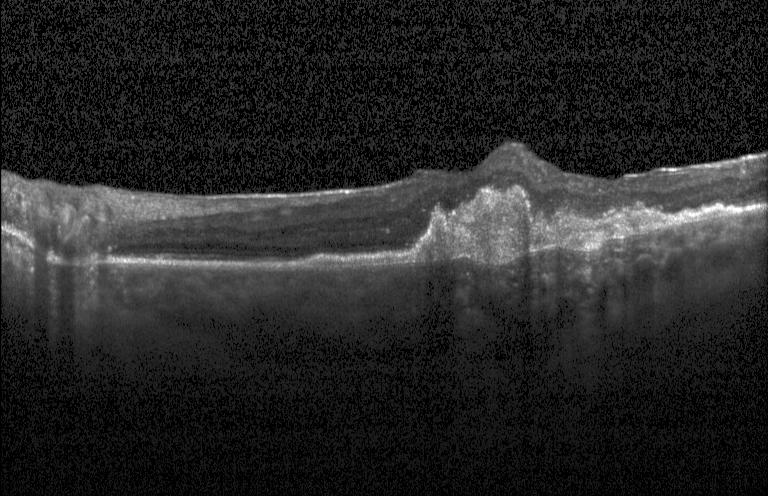 Finding: CNV.